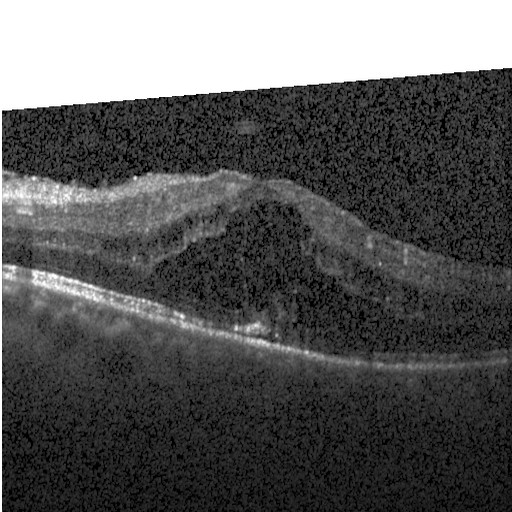
OCT scan showing diabetic macular edema.